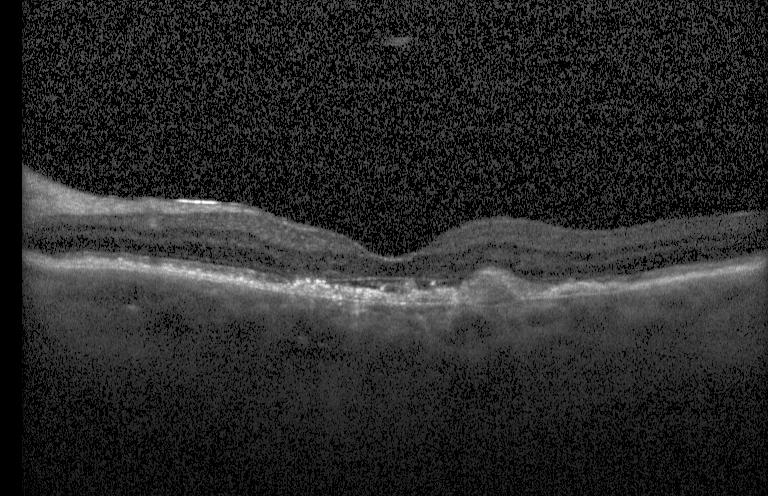 This B-scan demonstrates a choroidal neovascular membrane.